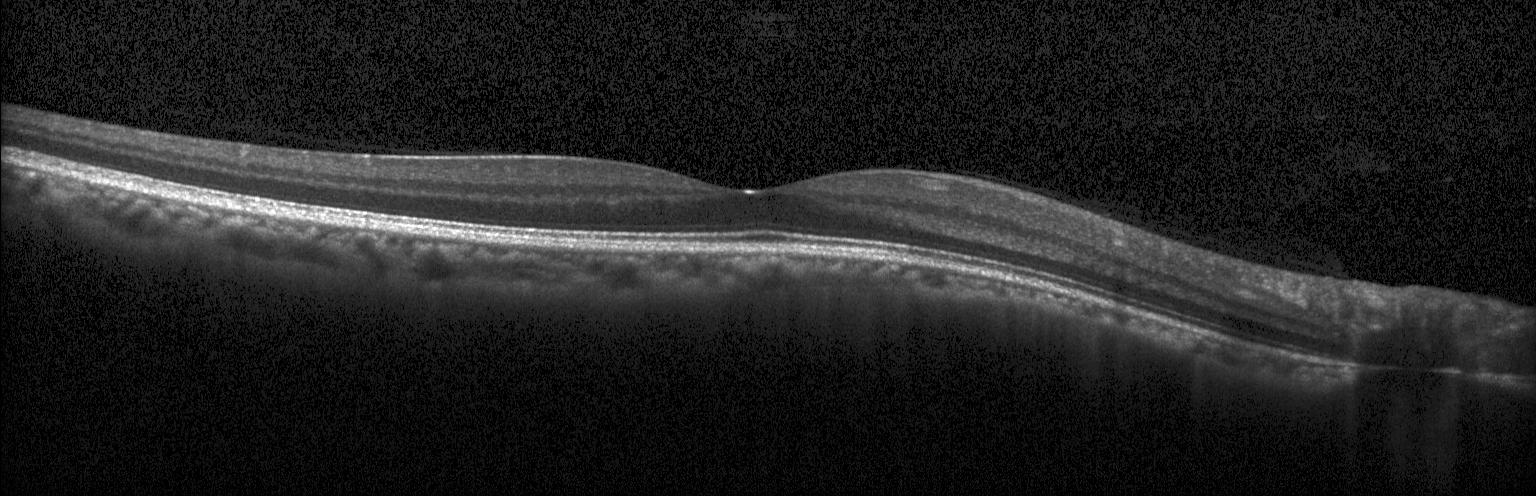 OCT line scan — Diagnosis: no choroidal neovascularization, no diabetic macular edema, and no drusen.